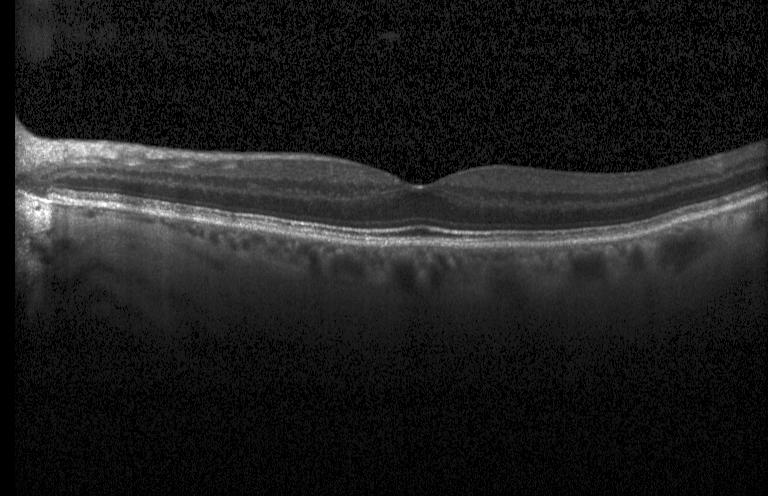
OCT line scan — Dx: no evidence of CNV, DME, or drusen.